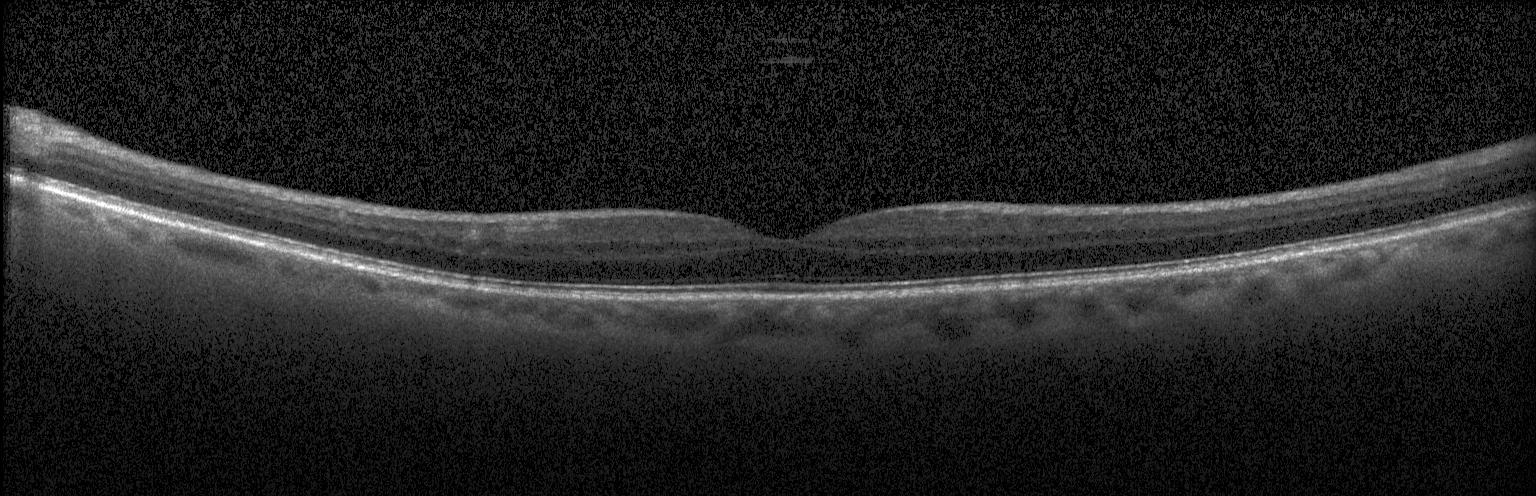 This B-scan demonstrates no choroidal neovascularization, no diabetic macular edema, and no drusen.